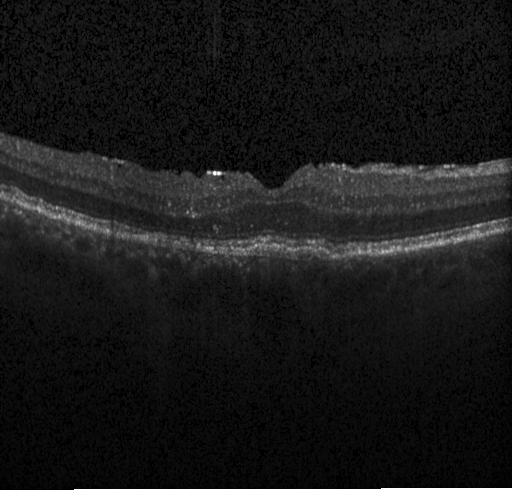

SD-OCT · retinal OCT B-scan · fovea-centered · Heidelberg Spectralis OCT system
The scan shows a choroidal neovascular membrane.